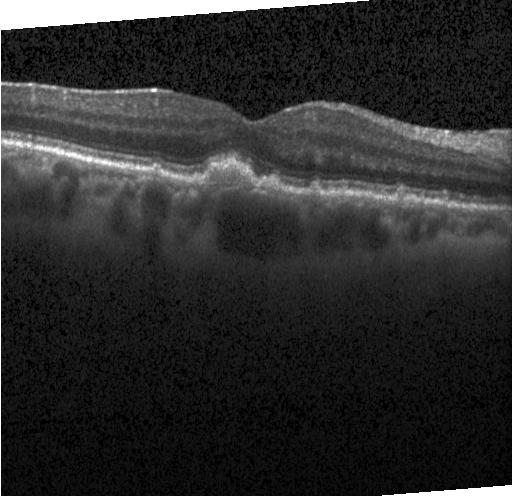 Retinal OCT B-scan · acquired on a Heidelberg Spectralis
The scan shows sub-RPE drusenoid deposits.